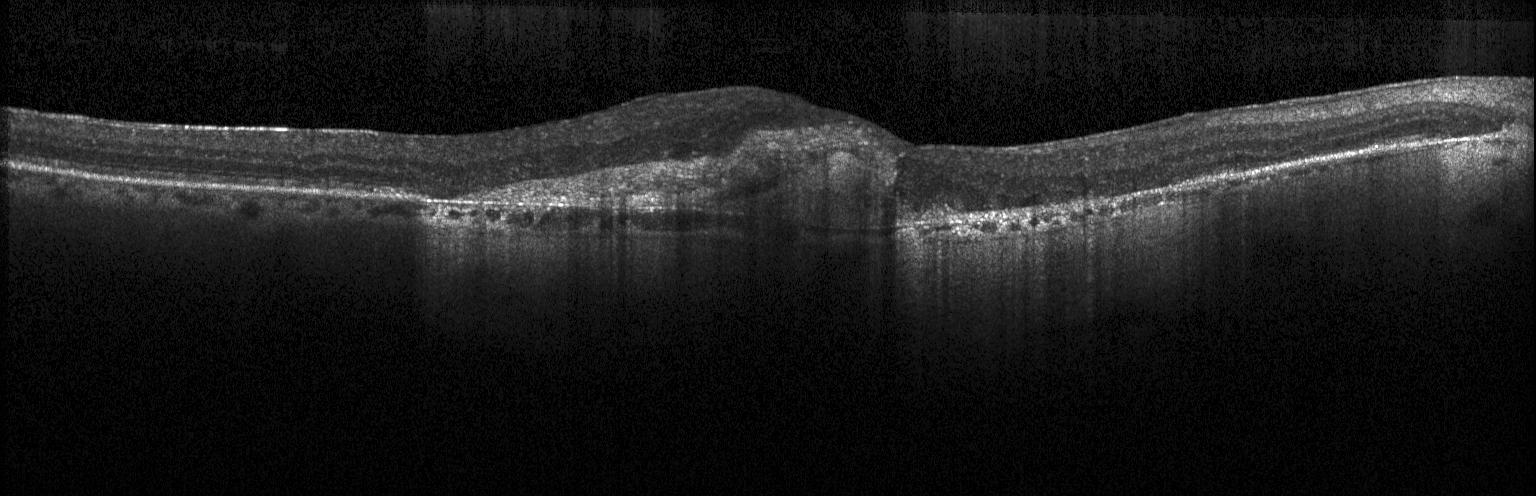
Spectral-domain OCT B-scan: a choroidal neovascular membrane.